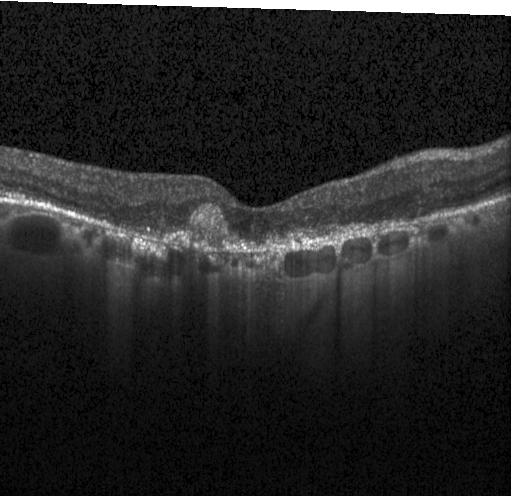 Optical coherence tomography scan. Impression: a choroidal neovascular membrane.